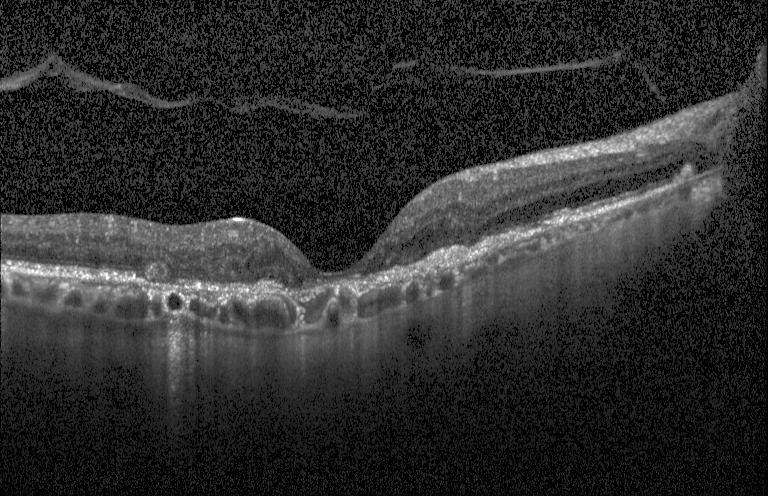

Impression: choroidal neovascularization (CNV).